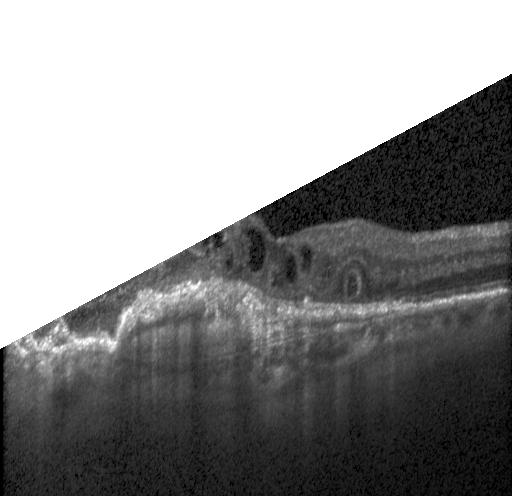
Finding: choroidal neovascularization (CNV).